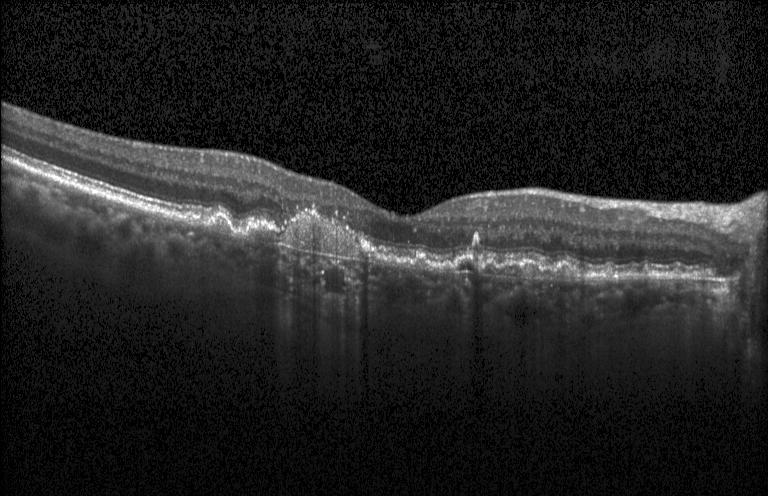

Retinal OCT B-scan — Diagnosis: a choroidal neovascular membrane.